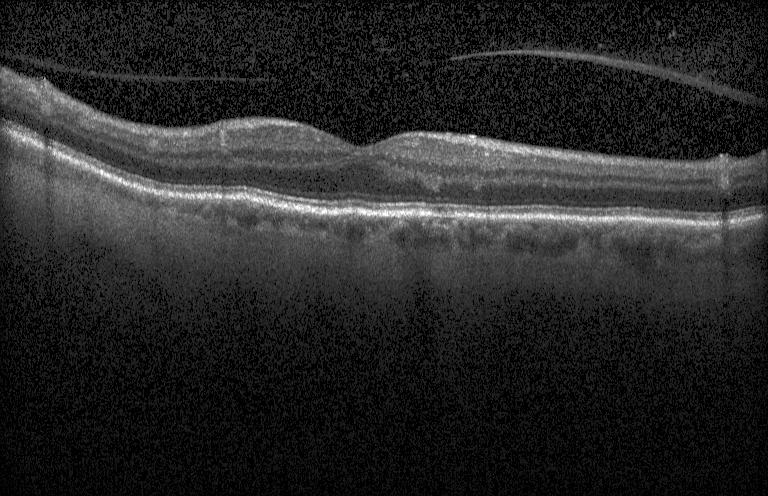
Retinal OCT B-scan. No CNV, DME, or drusen.